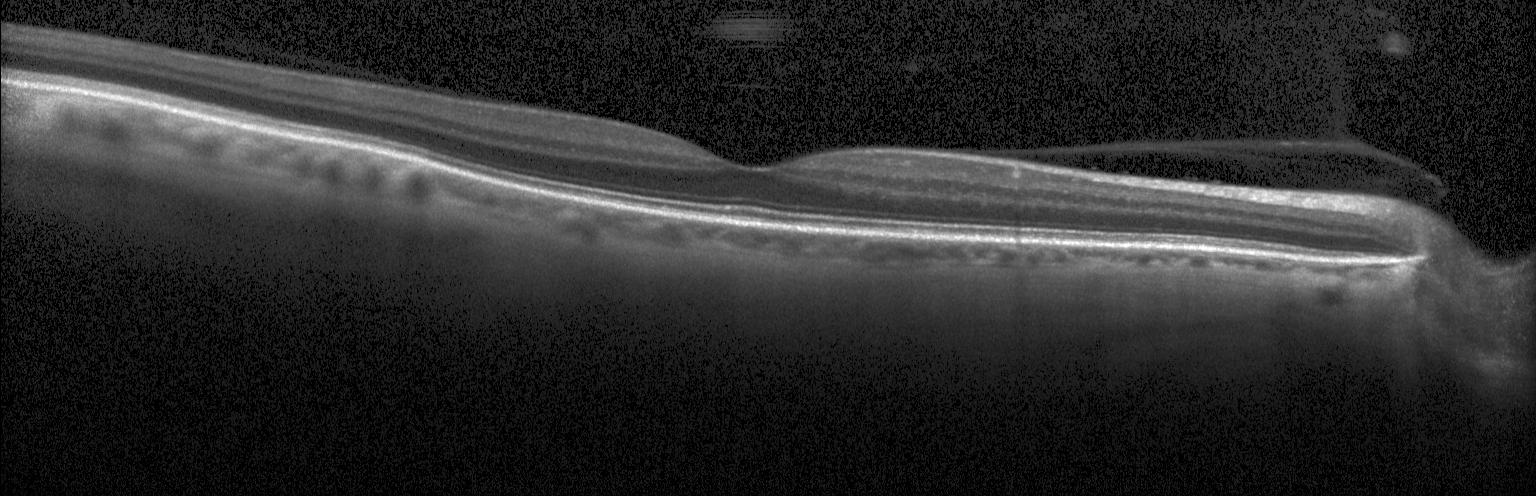 SD-OCT · optical coherence tomography B-scan · through the macula. This B-scan demonstrates neither CNV, DME, nor drusen.